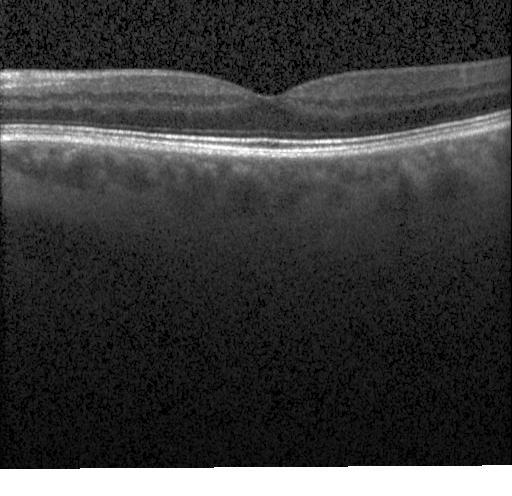
Spectral-domain OCT B-scan: no evidence of CNV, DME, or drusen.